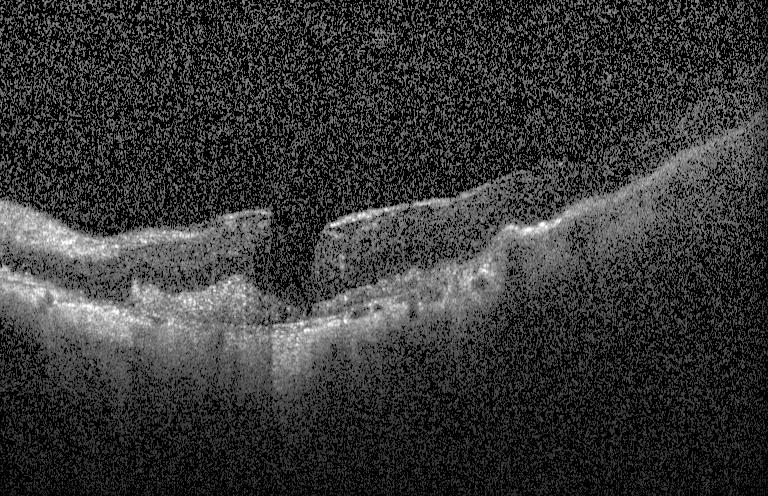 OCT B-scan showing choroidal neovascularization (CNV).